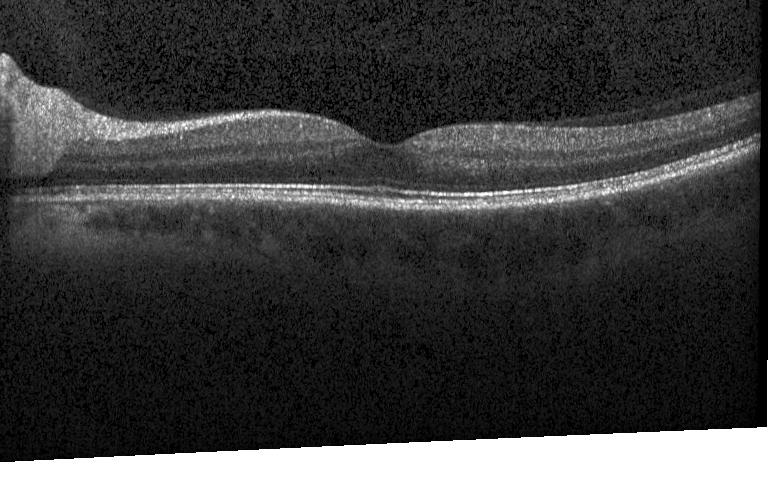

Through the macula. OCT B-scan. SD-OCT.
Finding: no evidence of choroidal neovascularization, diabetic macular edema, or drusen.